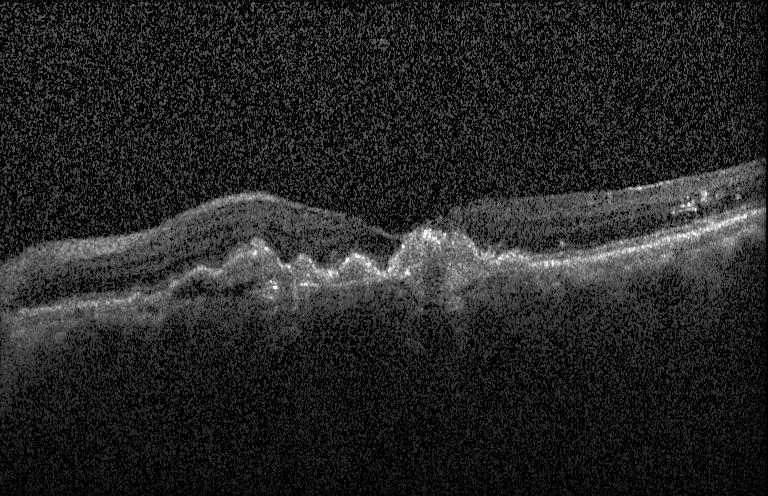 OCT B-scan. Acquired on a Heidelberg Spectralis
The scan shows a choroidal neovascular membrane.